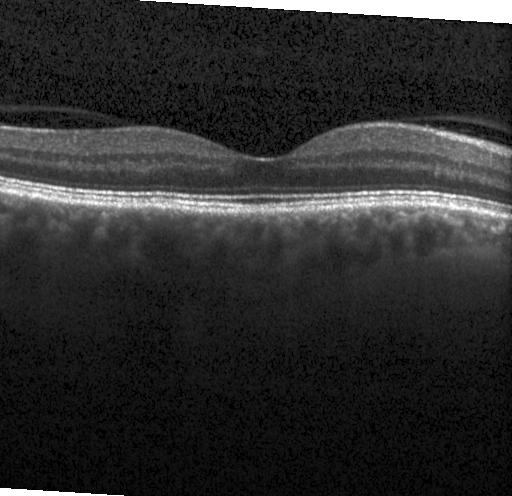
Dx: no CNV, DME, or drusen.